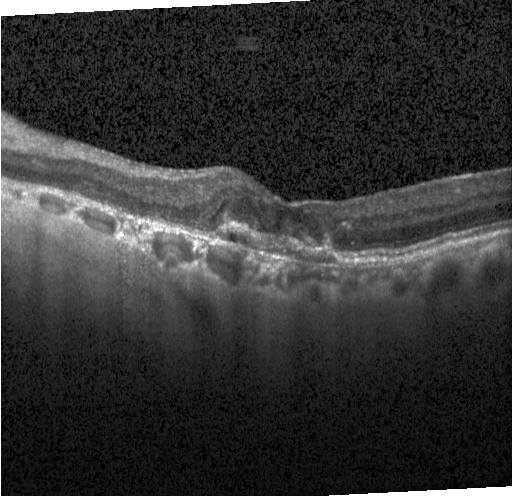 Optical coherence tomography B-scan · acquired on a Heidelberg Spectralis. A choroidal neovascular membrane.